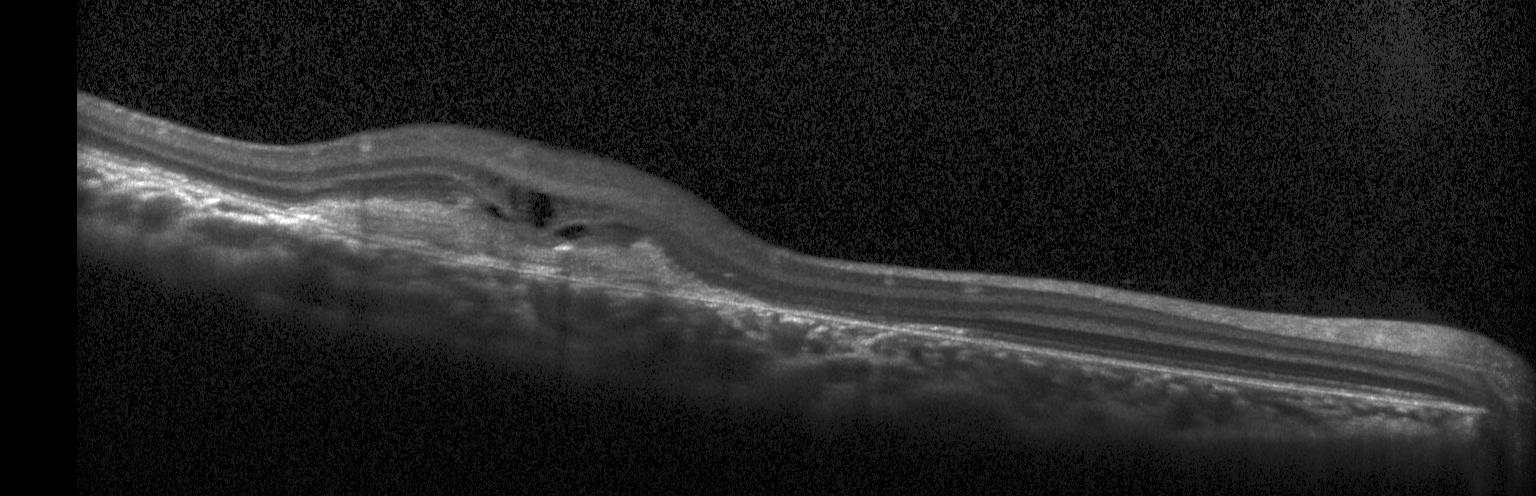

Spectral-domain optical coherence tomography; OCT B-scan; centered on the fovea; instrument: Heidelberg Spectralis
Macular OCT: choroidal neovascularization.